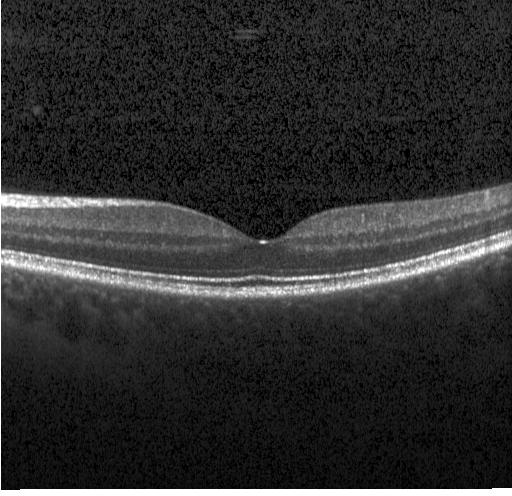 OCT B-scan — No choroidal neovascularization, diabetic macular edema, or drusen.